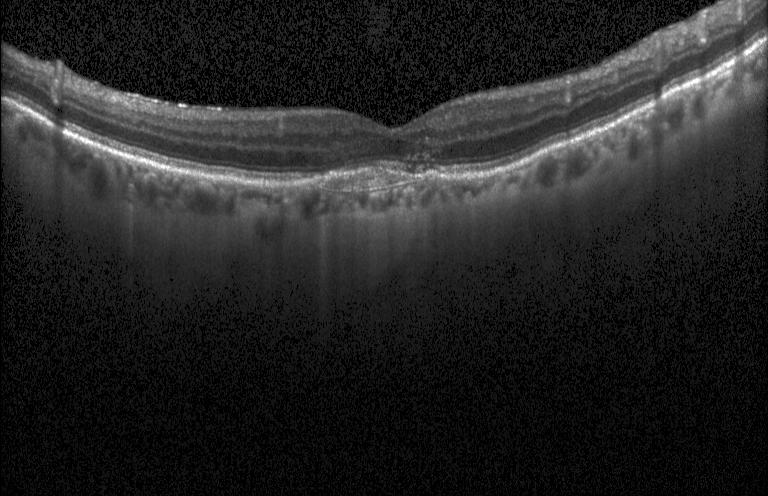
OCT scan showing a choroidal neovascular membrane.